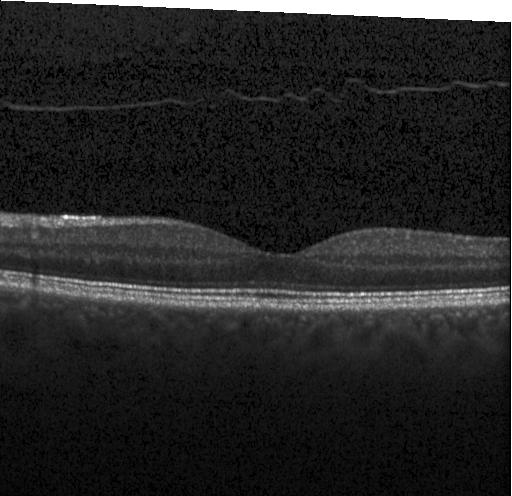
Spectral-domain OCT; acquired on a Heidelberg Spectralis; optical coherence tomography B-scan — Diagnosis: no choroidal neovascularization, no diabetic macular edema, and no drusen.